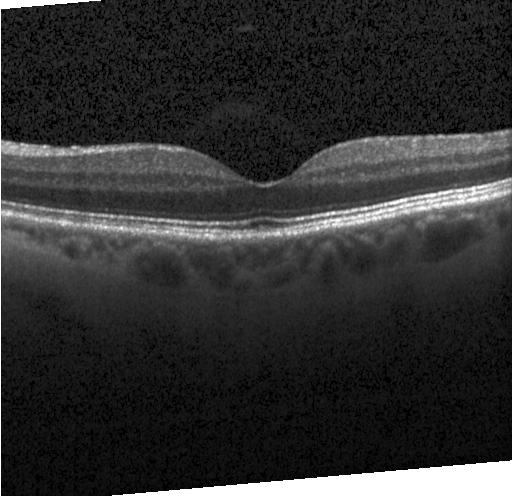

Assessment: no evidence of choroidal neovascularization, diabetic macular edema, or drusen.